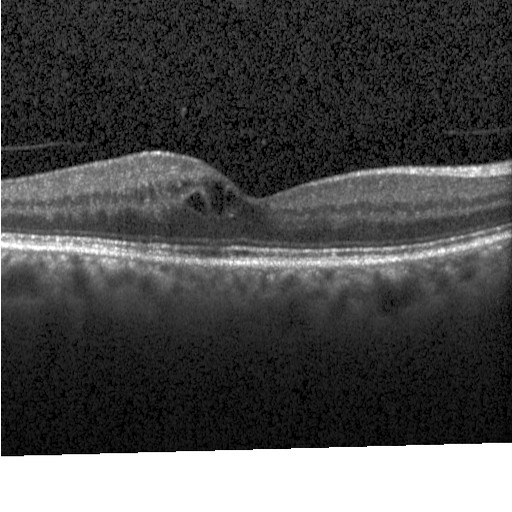
Retinal OCT cross-section — OCT finding: diabetic macular edema (DME).